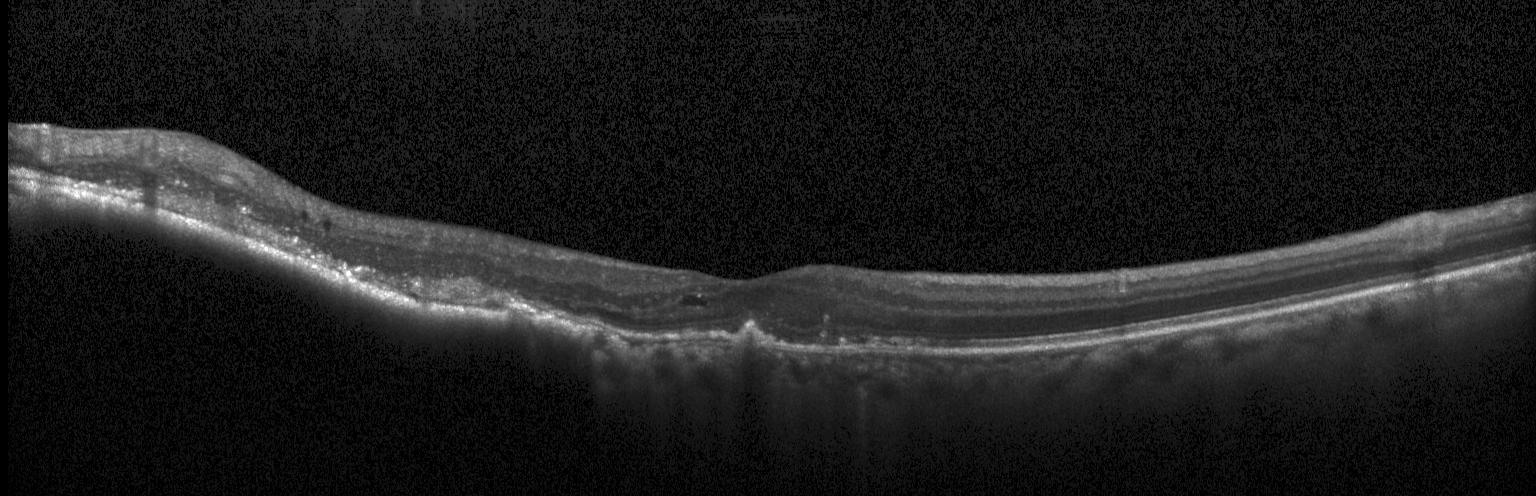

Assessment: CNV.